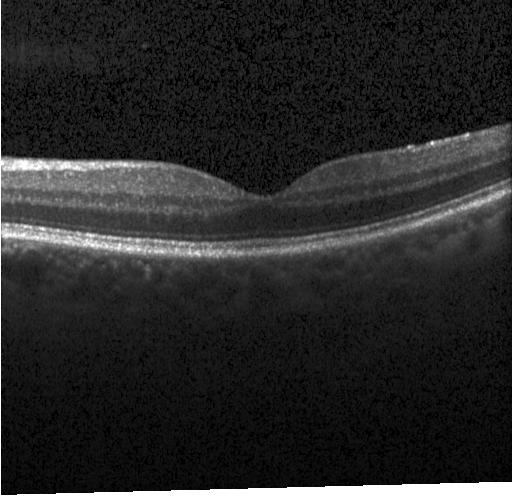 Retinal OCT cross-section.
Impression: neither CNV, DME, nor drusen.